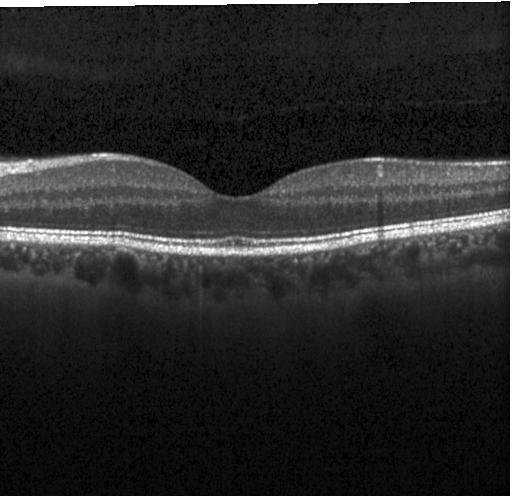 Spectral-domain optical coherence tomography · retinal OCT cross-section · Heidelberg Spectralis OCT system · fovea-centered — Impression: no choroidal neovascularization, diabetic macular edema, or drusen.